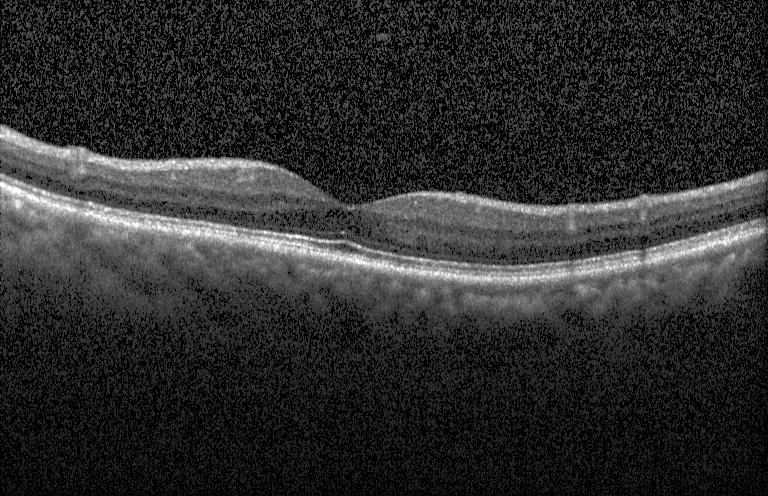

Centered on the fovea, spectral-domain optical coherence tomography, OCT line scan — Assessment: no evidence of choroidal neovascularization, diabetic macular edema, or drusen.